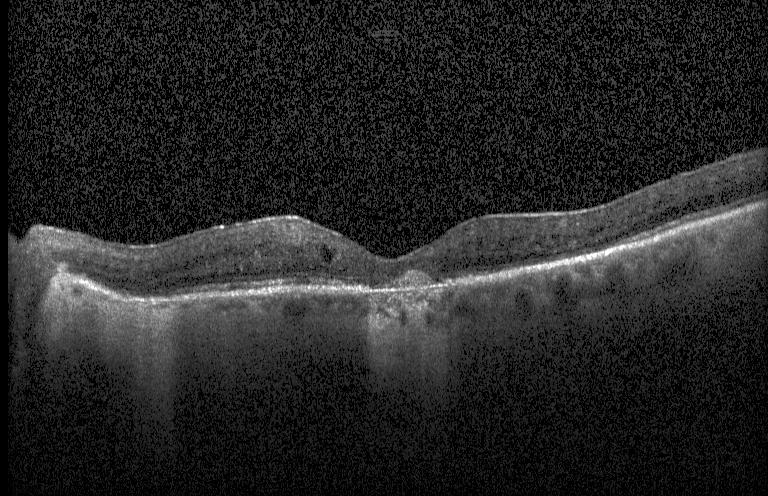

OCT B-scan.
Finding: a choroidal neovascular membrane.